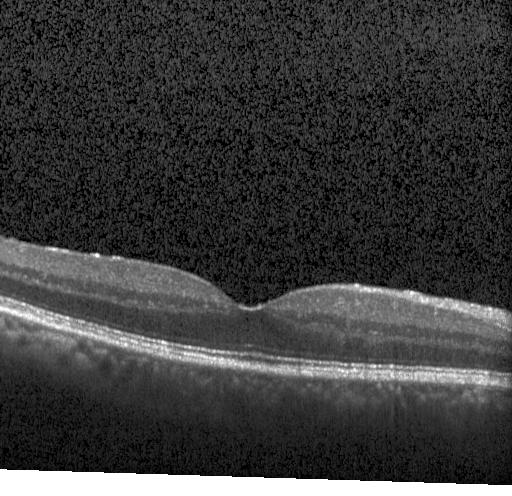 Impression: no choroidal neovascularization, no diabetic macular edema, and no drusen.